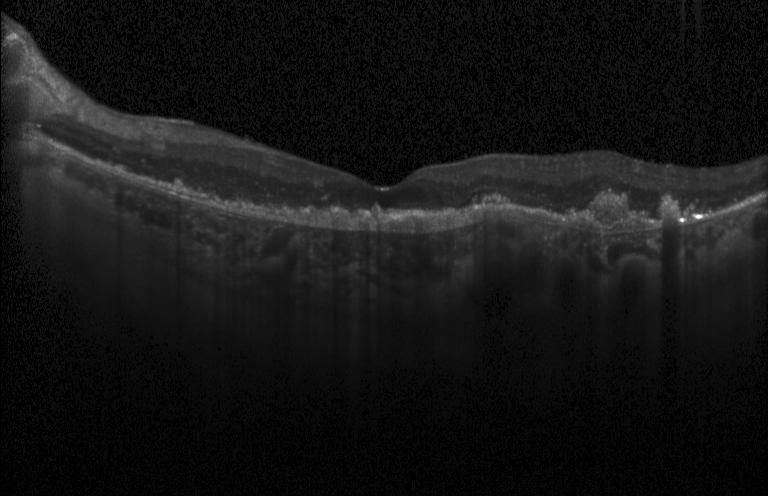 Diagnosis: a choroidal neovascular membrane.